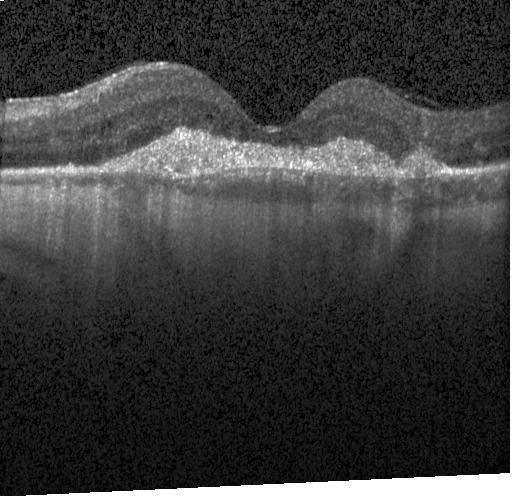
Centered on the fovea. Spectral-domain OCT. OCT B-scan — Diagnosis: a choroidal neovascular membrane.